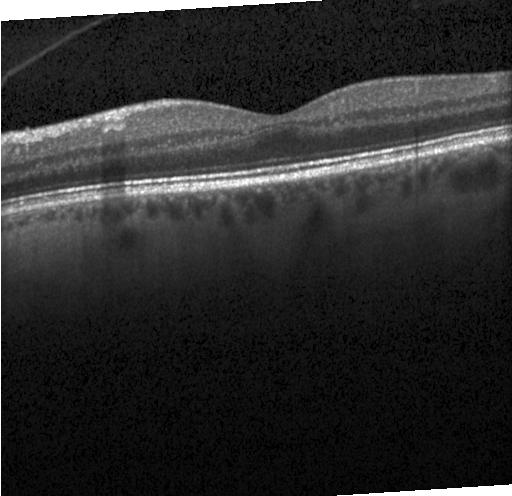
Retinal OCT cross-section showing no choroidal neovascularization, no diabetic macular edema, and no drusen.